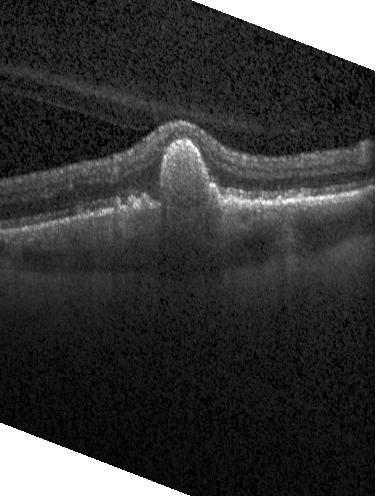
Fovea-centered, OCT B-scan, Heidelberg Spectralis OCT system, SD-OCT — OCT finding: a choroidal neovascular membrane.